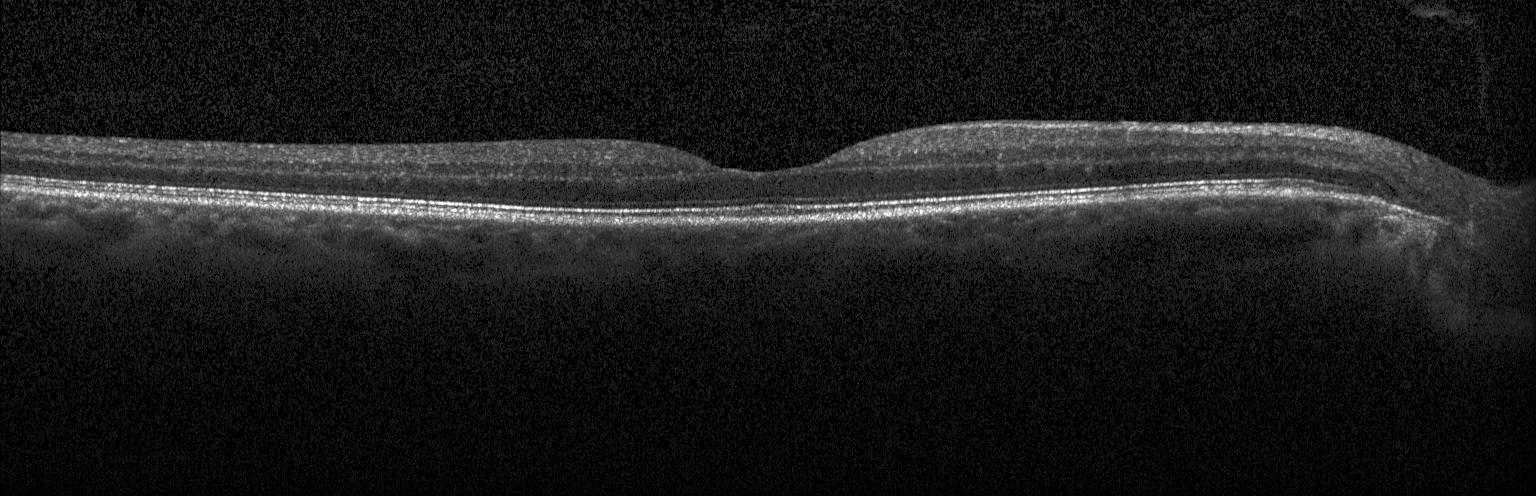 Diagnosis: no CNV, DME, or drusen.